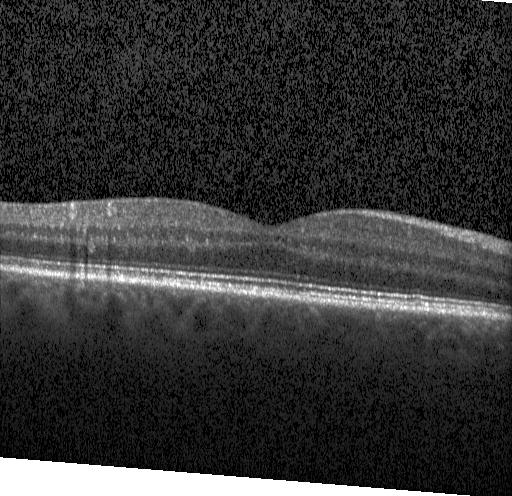 Retinal OCT cross-section. Heidelberg Spectralis — OCT finding: no choroidal neovascularization, diabetic macular edema, or drusen.